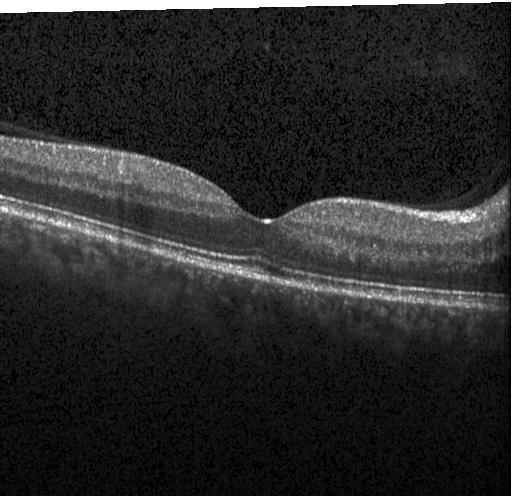
This B-scan demonstrates no choroidal neovascularization, no diabetic macular edema, and no drusen.